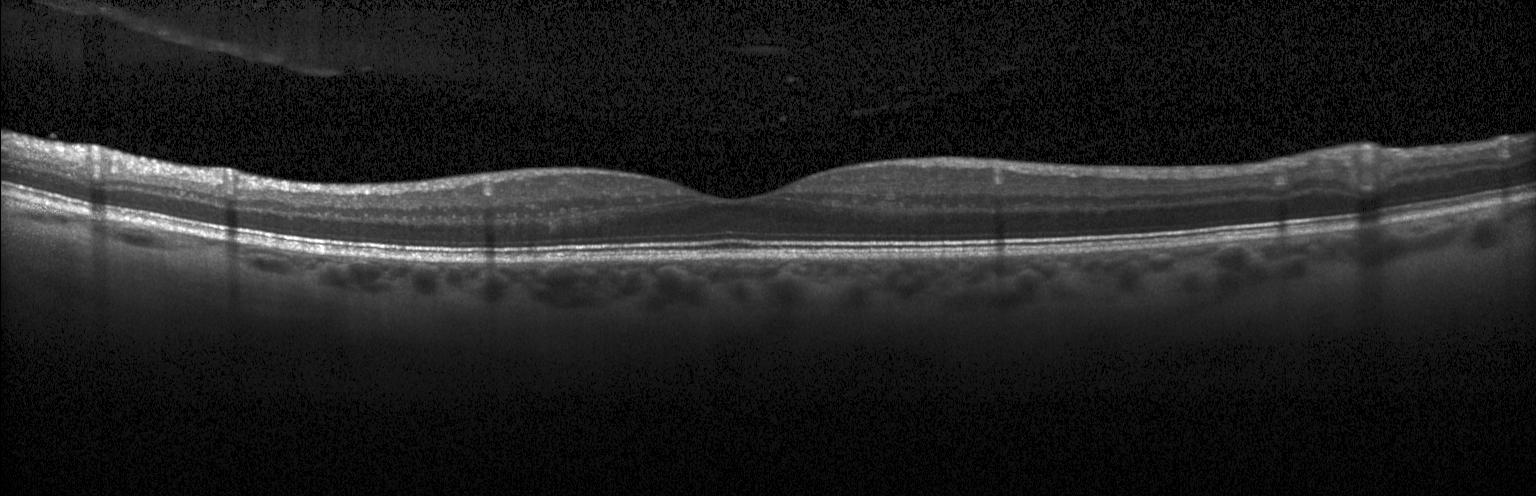
Spectral-domain OCT B-scan: no evidence of choroidal neovascularization, diabetic macular edema, or drusen.